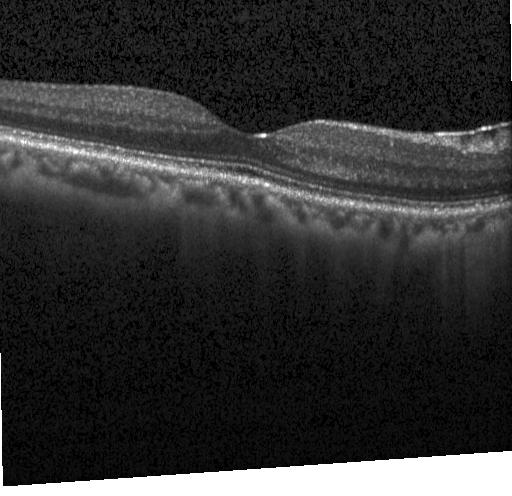

Retinal OCT B-scan; spectral-domain optical coherence tomography; horizontal scan through the fovea. No evidence of choroidal neovascularization, diabetic macular edema, or drusen.